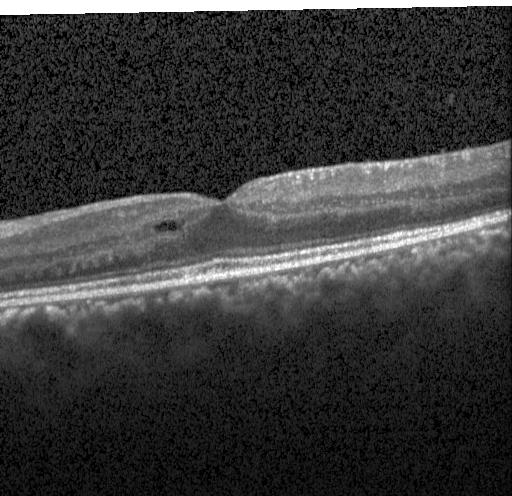
Spectral-domain optical coherence tomography. Heidelberg Spectralis. Retinal OCT B-scan. Fovea-centered
Diagnosis: diabetic macular edema.